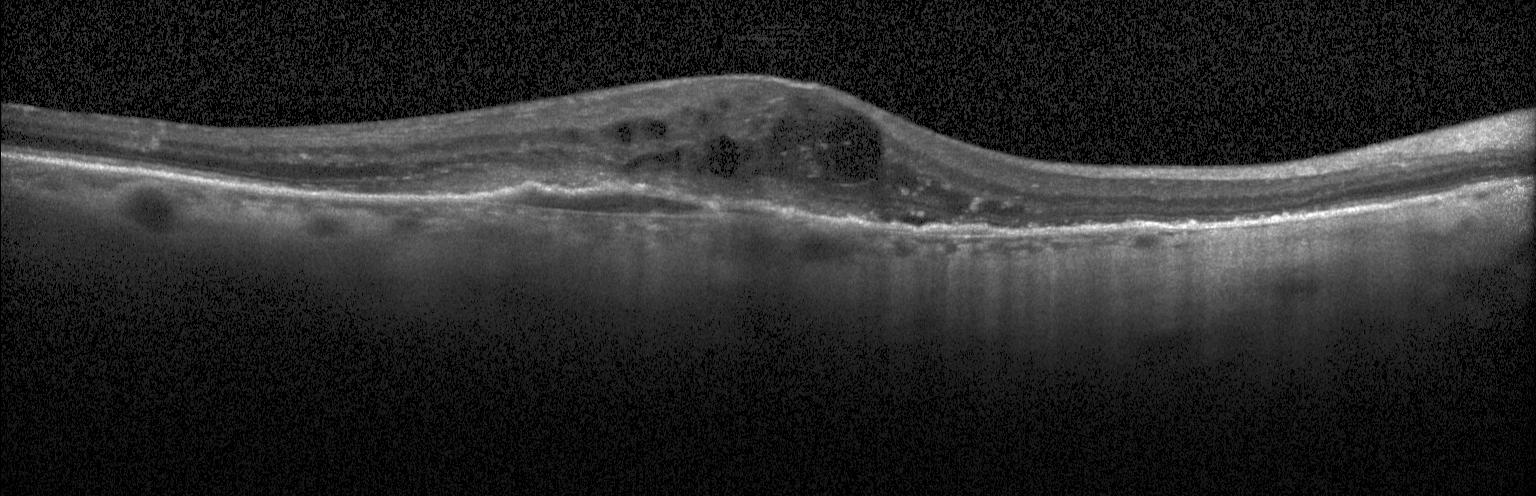

Spectral-domain optical coherence tomography, macular scan, OCT B-scan, Heidelberg Spectralis — The scan shows choroidal neovascularization.